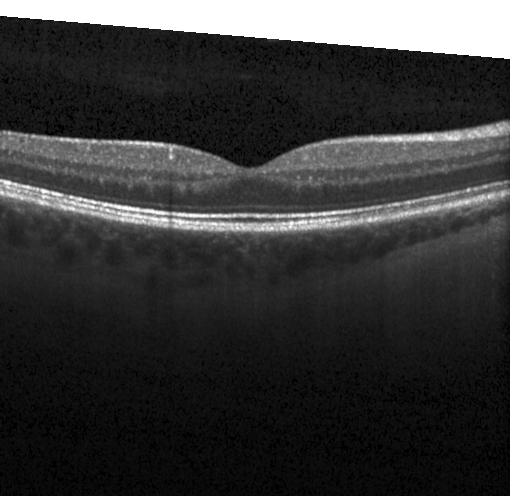

Spectral-domain OCT. Retinal OCT B-scan. Heidelberg Spectralis OCT system. Centered on the fovea — The scan shows no choroidal neovascularization, diabetic macular edema, or drusen.